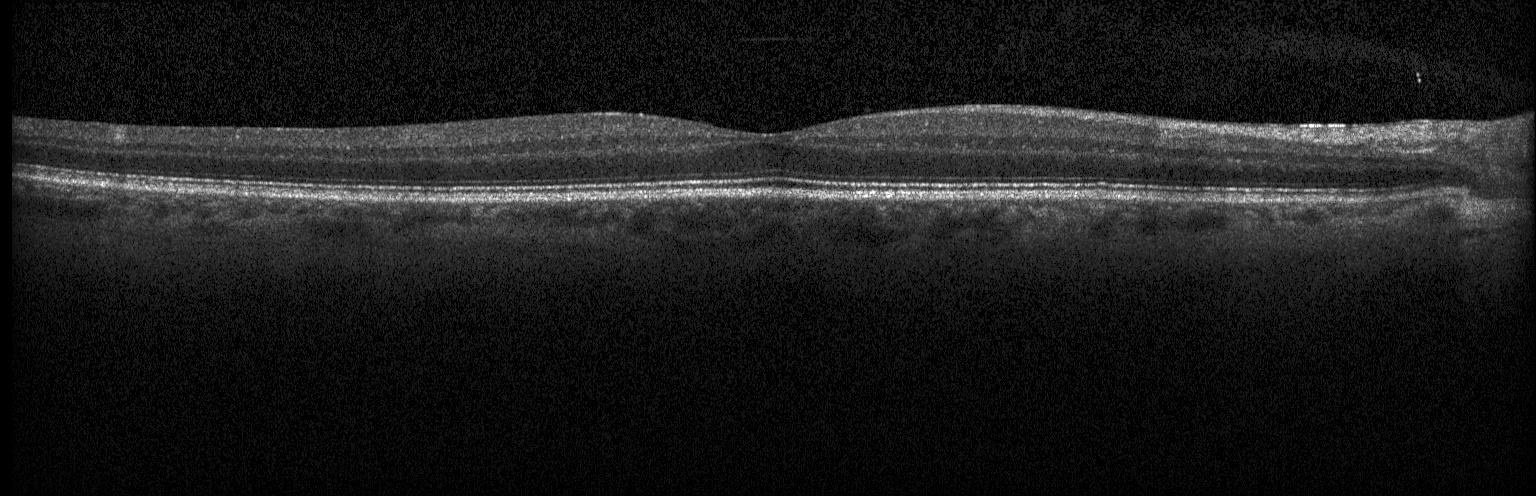
SD-OCT, Heidelberg Spectralis OCT system, horizontal scan through the fovea, retinal OCT B-scan. The scan shows no evidence of CNV, DME, or drusen.